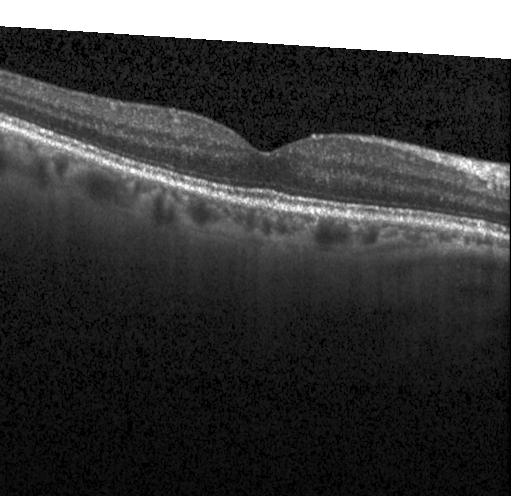

Impression: no evidence of choroidal neovascularization, diabetic macular edema, or drusen.